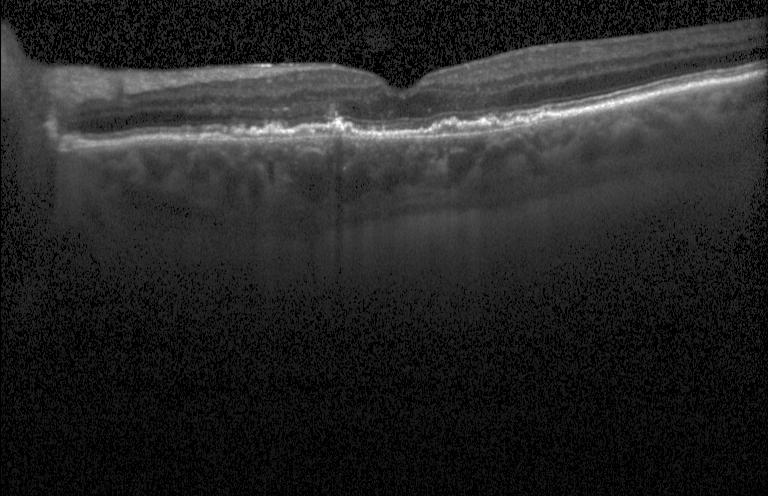

Finding: choroidal neovascularization (CNV).